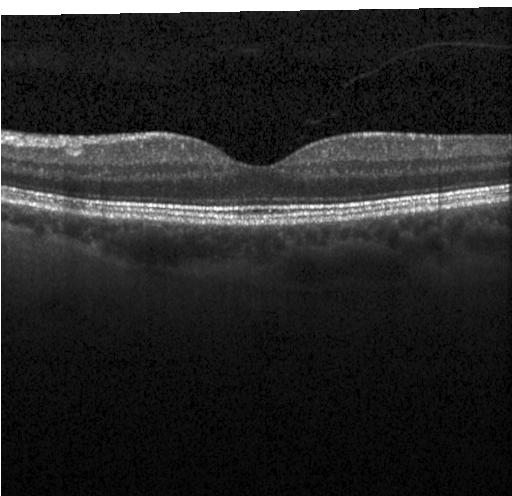 Diagnosis: no CNV, DME, or drusen.